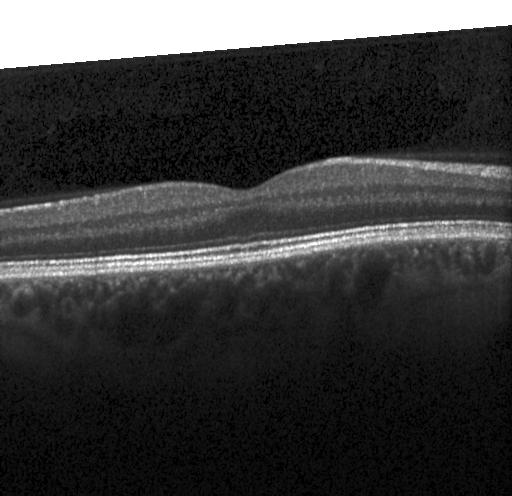

OCT finding: no evidence of choroidal neovascularization, diabetic macular edema, or drusen.